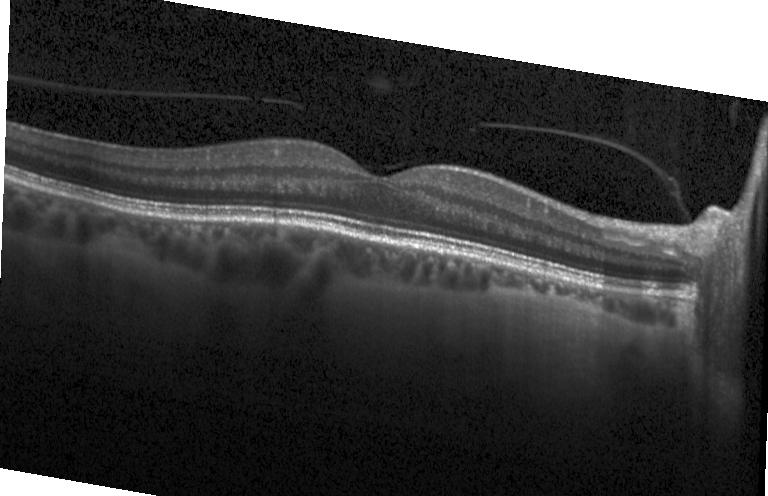

Macular scan, acquired on a Heidelberg Spectralis, spectral-domain OCT, retinal OCT cross-section.
Finding: no choroidal neovascularization, no diabetic macular edema, and no drusen.